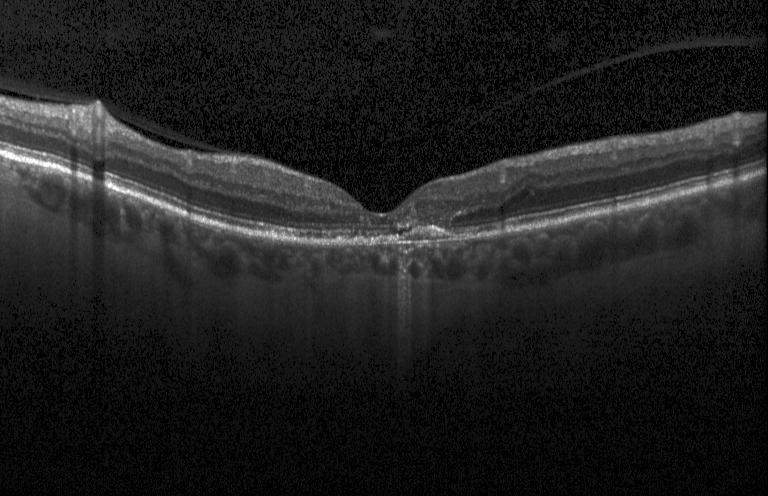 Optical coherence tomography scan — A choroidal neovascular membrane.